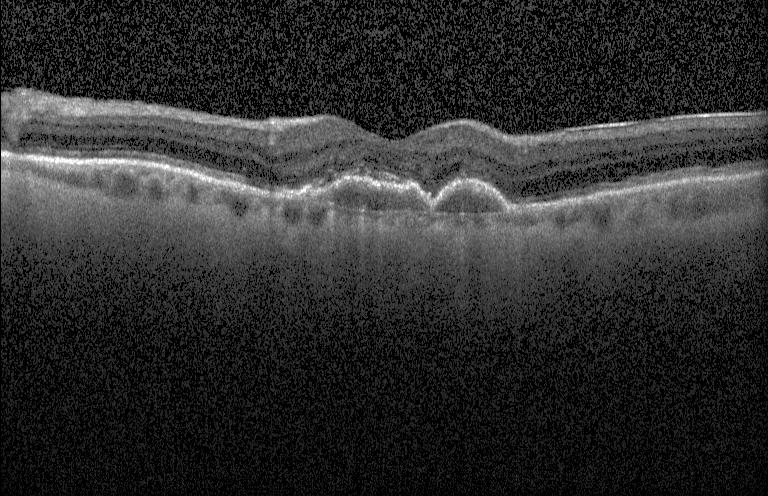 Finding: a choroidal neovascular membrane.